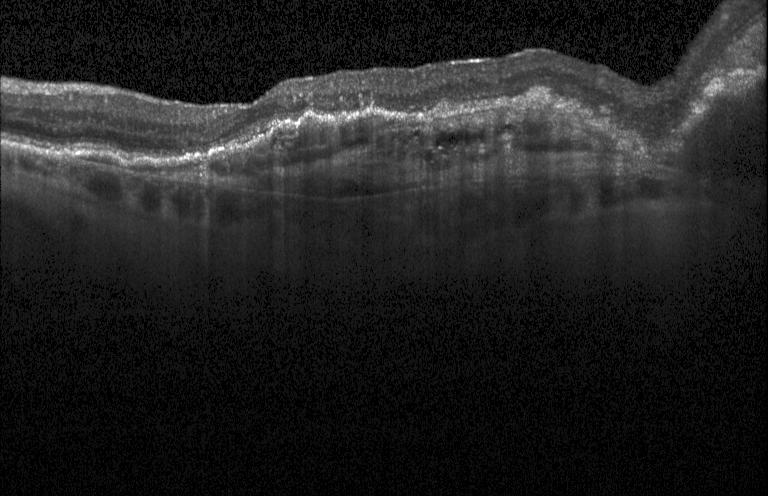

Fovea-centered, SD-OCT, OCT B-scan. Assessment: choroidal neovascularization.